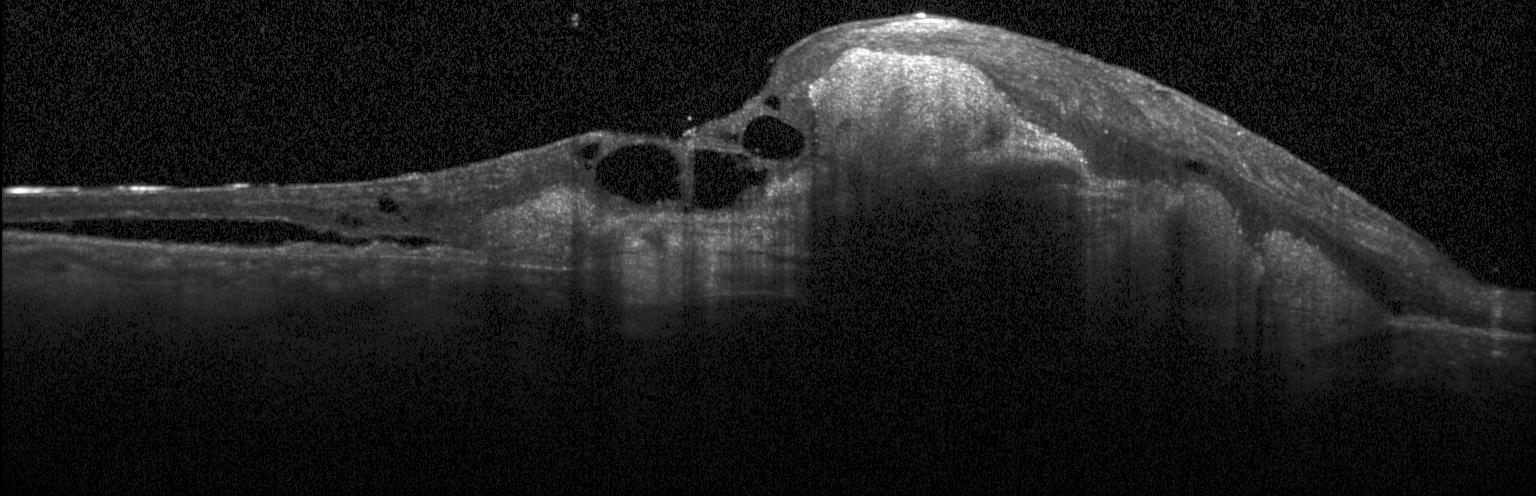
Spectral-domain OCT, Heidelberg Spectralis, OCT line scan. Diagnosis: a choroidal neovascular membrane.